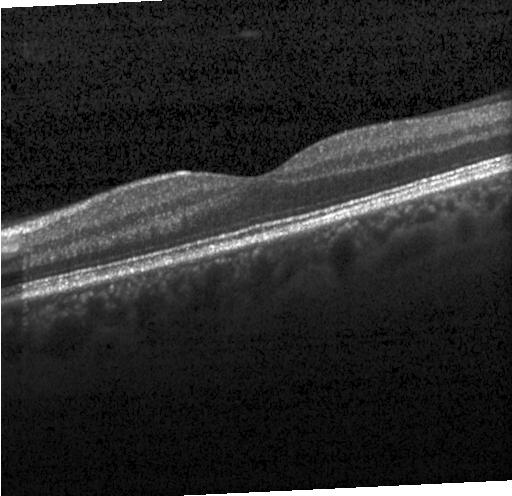

Fovea-centered, spectral-domain OCT, retinal OCT cross-section, instrument: Heidelberg Spectralis — The scan shows no CNV, DME, or drusen.